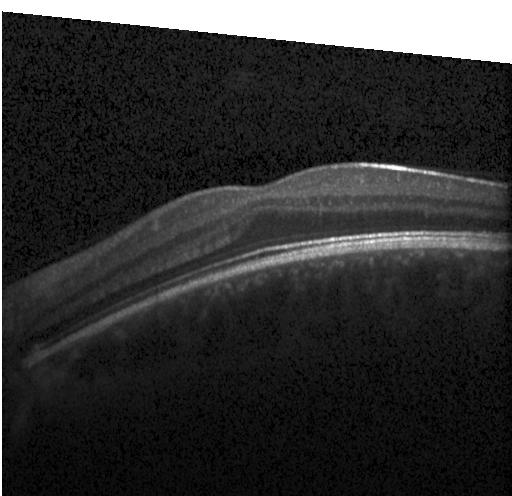
Heidelberg Spectralis, horizontal scan through the fovea, SD-OCT, OCT line scan — OCT finding: no evidence of choroidal neovascularization, diabetic macular edema, or drusen.